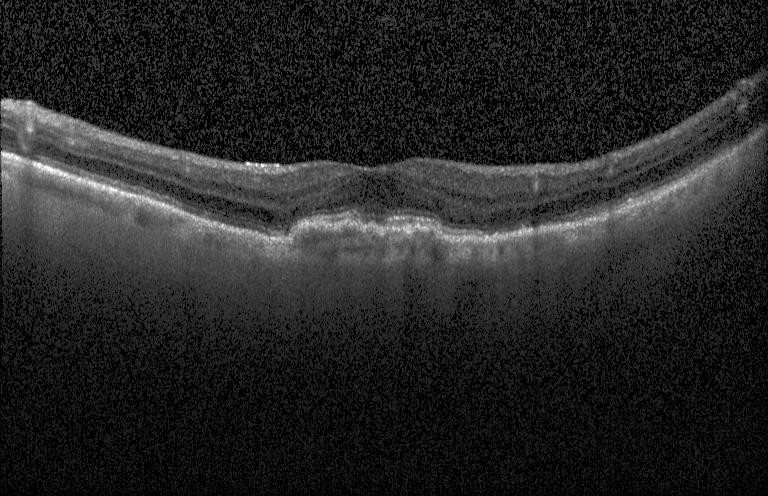
OCT B-scan. Heidelberg Spectralis OCT system. Through the macula. SD-OCT — Impression: a choroidal neovascular membrane.